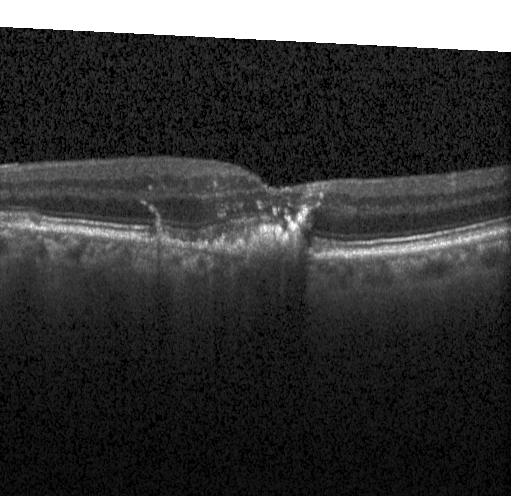

Assessment: a choroidal neovascular membrane.